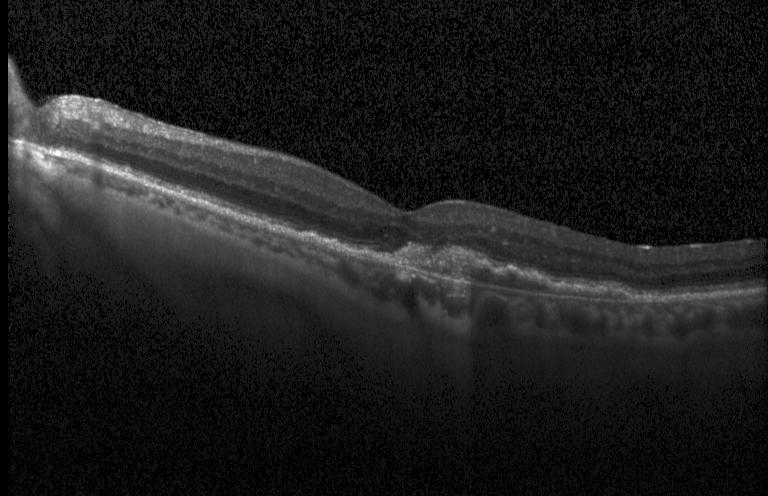
Heidelberg Spectralis OCT system. Through the macula. Optical coherence tomography B-scan. Spectral-domain OCT.
The scan shows a choroidal neovascular membrane.